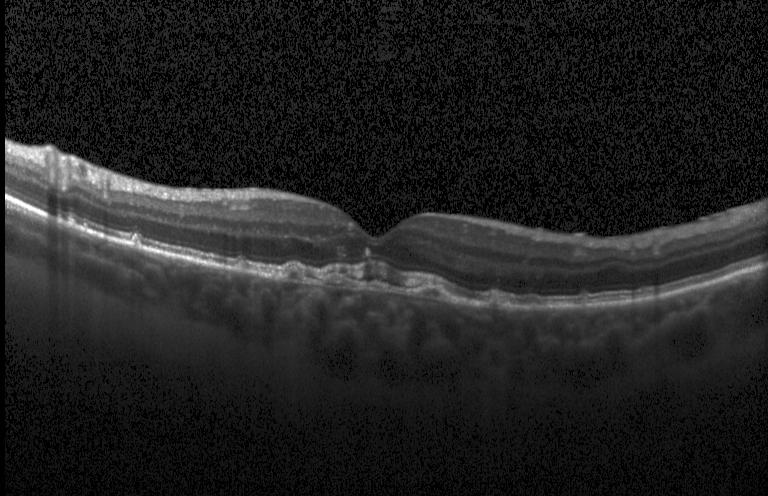
Diagnosis: a choroidal neovascular membrane.